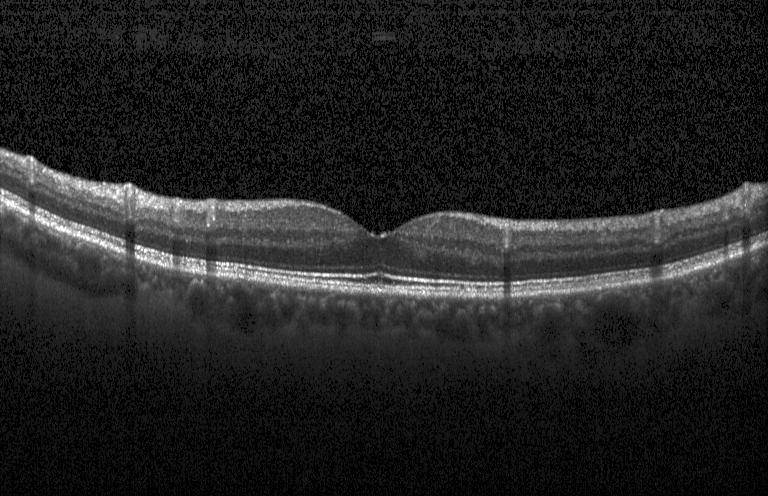 Centered on the fovea, optical coherence tomography scan, spectral-domain OCT
Assessment: no choroidal neovascularization, diabetic macular edema, or drusen.